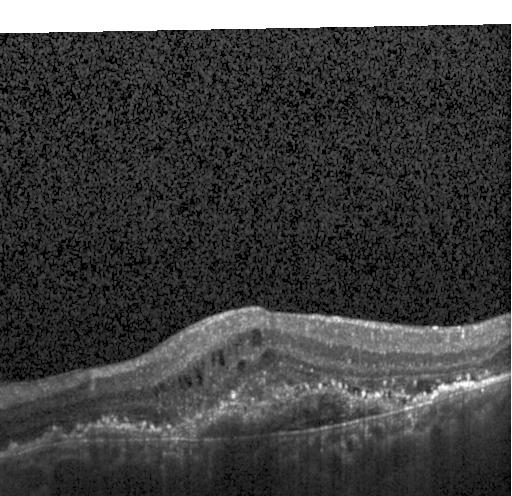 Spectral-domain OCT, optical coherence tomography B-scan, macular scan.
This B-scan demonstrates a choroidal neovascular membrane.